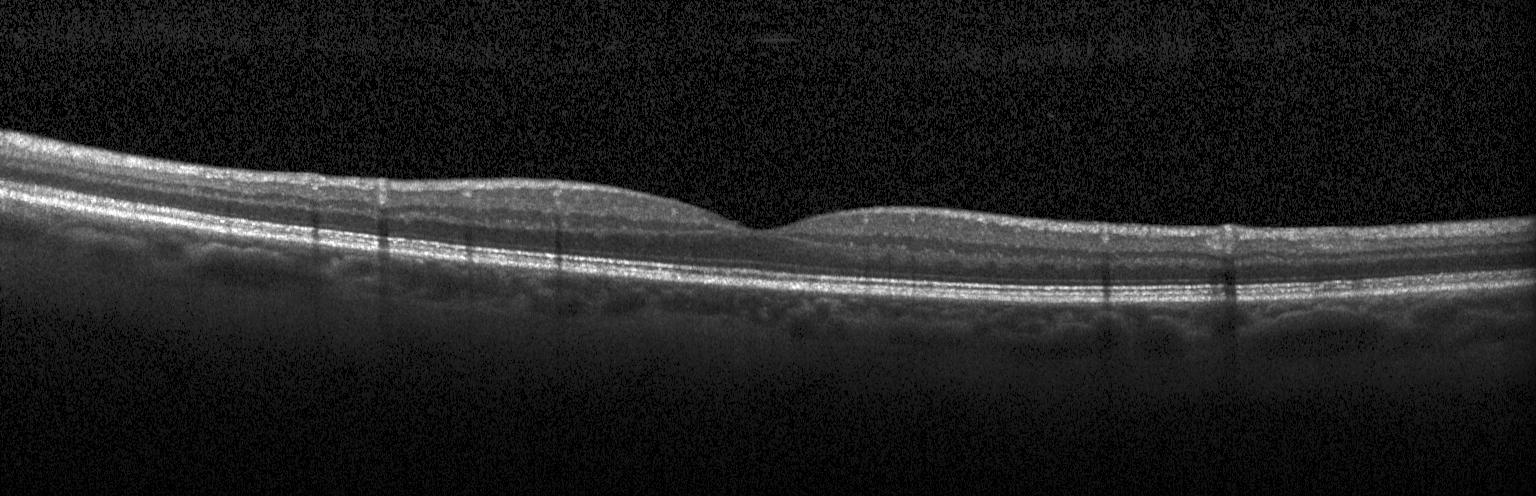

Dx: neither CNV, DME, nor drusen.